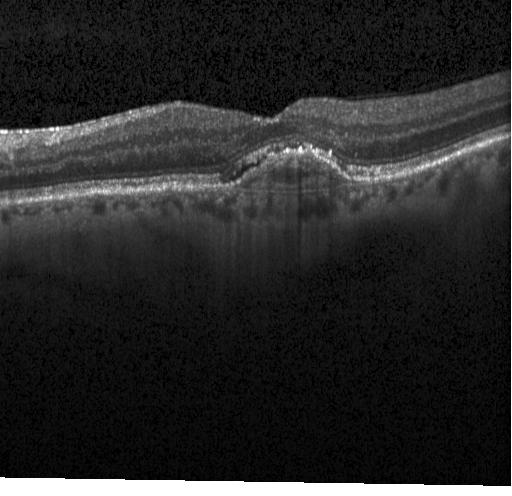
Retinal OCT B-scan — Impression: CNV.